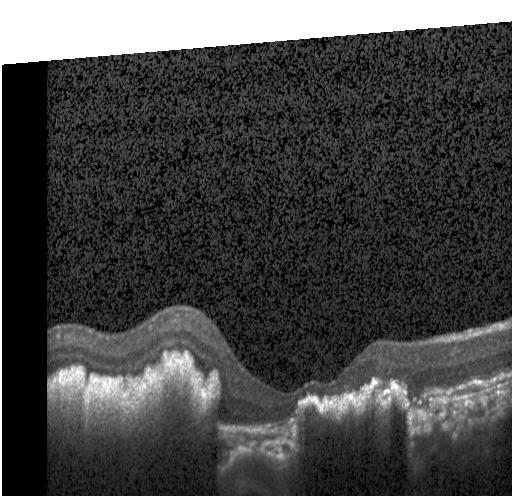
Optical coherence tomography B-scan, instrument: Heidelberg Spectralis — The scan shows choroidal neovascularization.